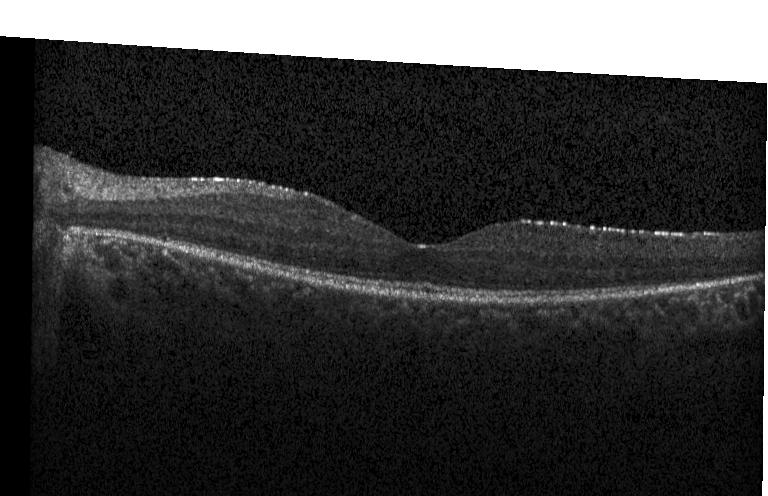

OCT B-scan. Neither choroidal neovascularization, diabetic macular edema, nor drusen.